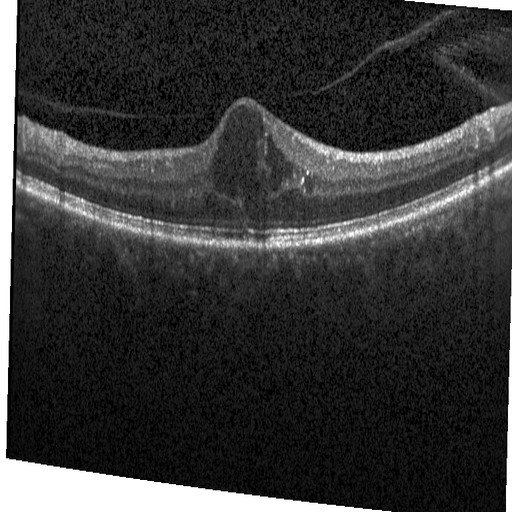
OCT scan showing DME.